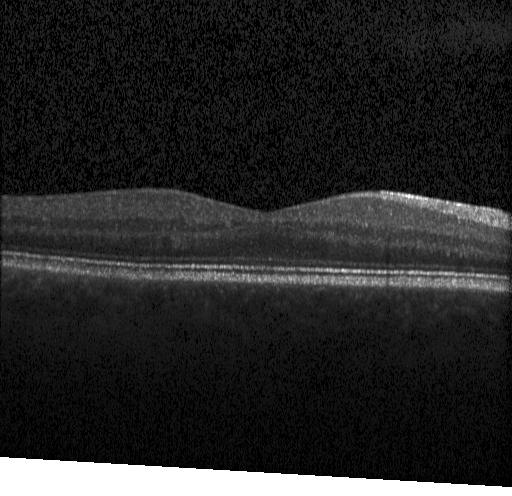
Heidelberg Spectralis, retinal OCT B-scan.
Assessment: no choroidal neovascularization, no diabetic macular edema, and no drusen.